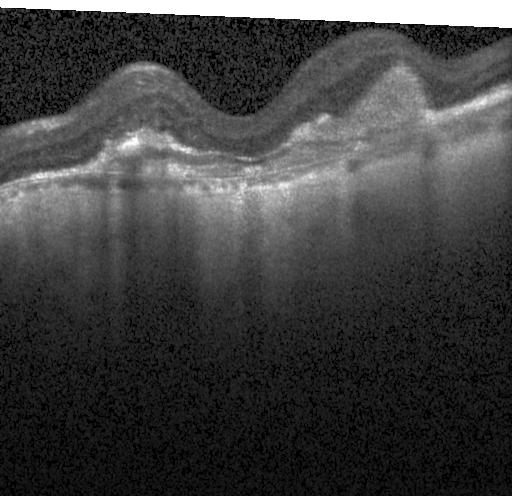
Horizontal scan through the fovea · OCT line scan. The scan shows a choroidal neovascular membrane.